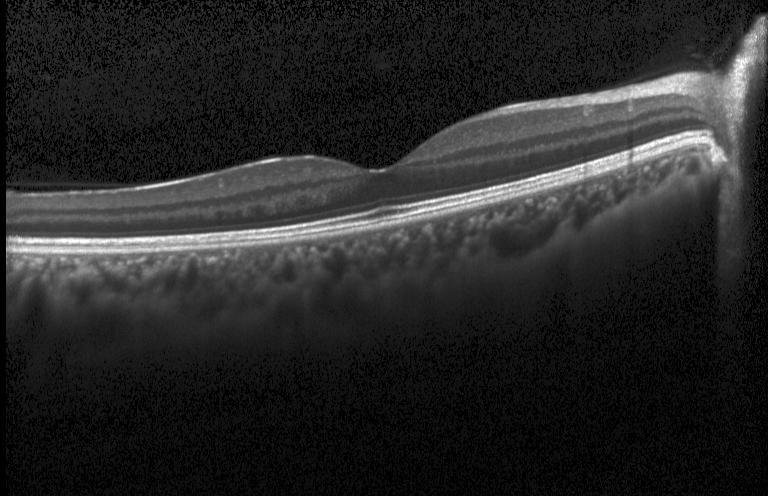

Diagnosis: no choroidal neovascularization, no diabetic macular edema, and no drusen.